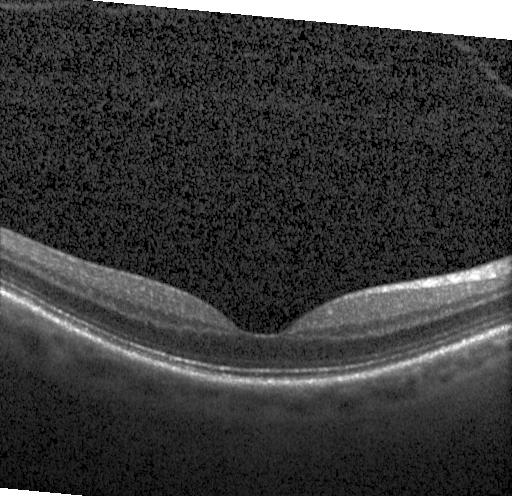

Diagnosis: no choroidal neovascularization, no diabetic macular edema, and no drusen.